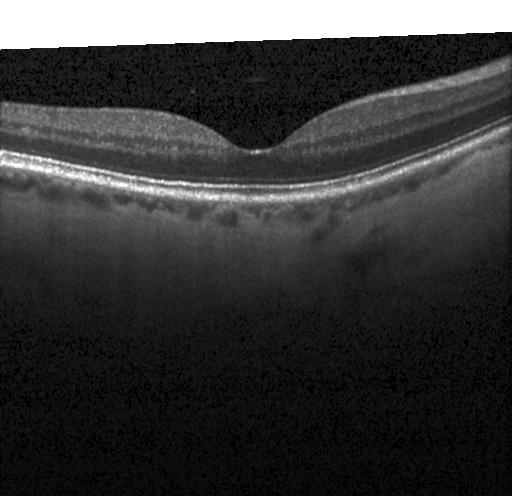
Fovea-centered. SD-OCT. OCT line scan
Diagnosis: neither choroidal neovascularization, diabetic macular edema, nor drusen.